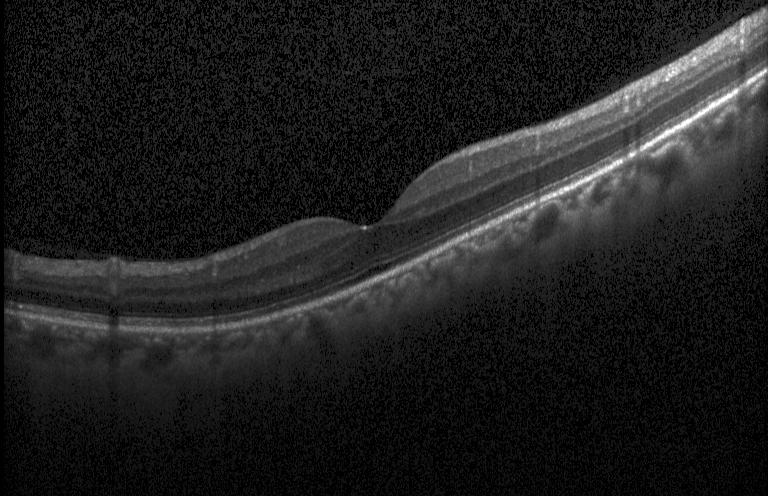
Heidelberg Spectralis. Optical coherence tomography scan. Macular scan
Diagnosis: neither choroidal neovascularization, diabetic macular edema, nor drusen.